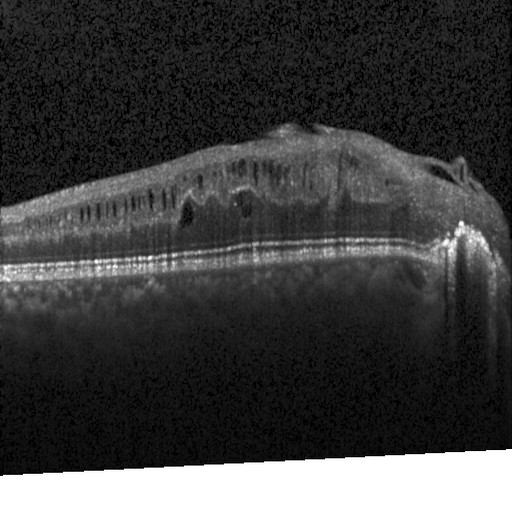
Retinal OCT B-scan; macular scan
Finding: DME.